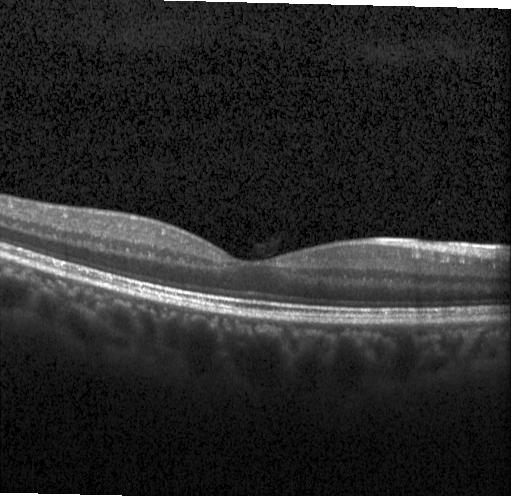

Acquired on a Heidelberg Spectralis, retinal OCT B-scan, SD-OCT, centered on the fovea.
Finding: neither choroidal neovascularization, diabetic macular edema, nor drusen.